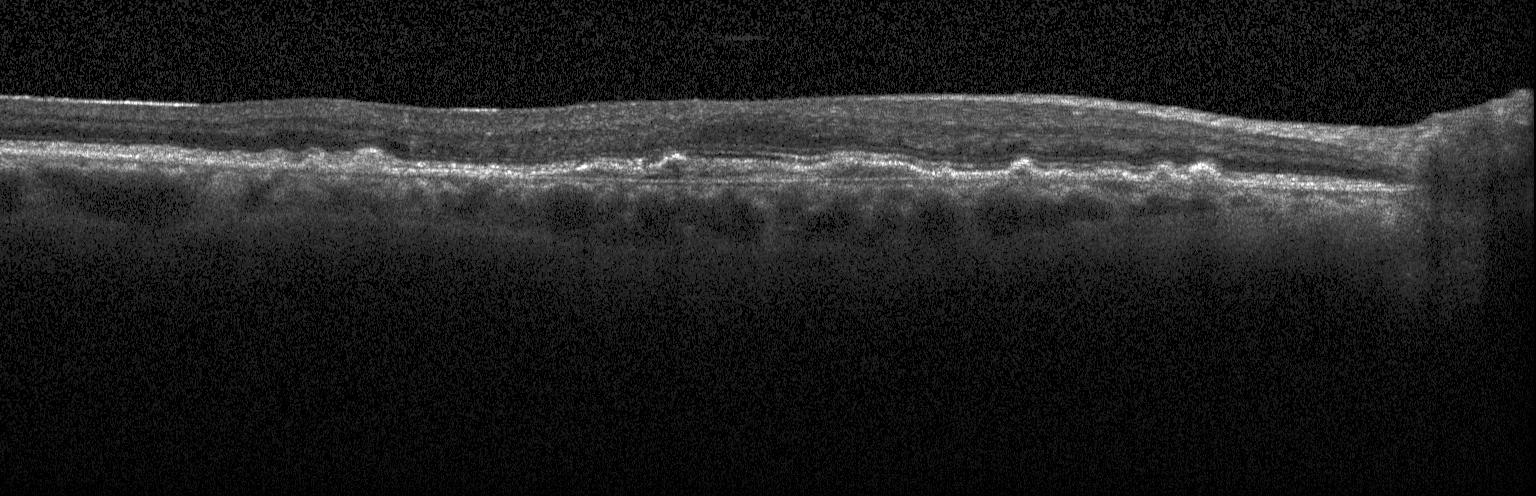

OCT B-scan — This B-scan demonstrates a choroidal neovascular membrane.